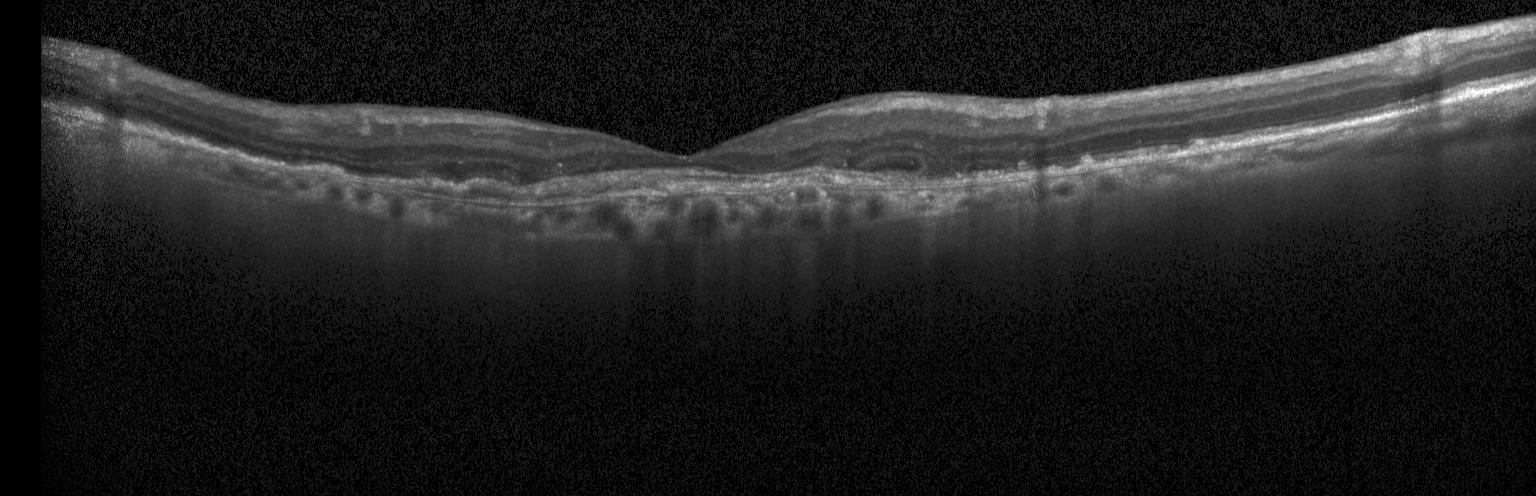

Heidelberg Spectralis OCT system, spectral-domain optical coherence tomography, through the macula, retinal OCT B-scan.
Assessment: choroidal neovascularization (CNV).